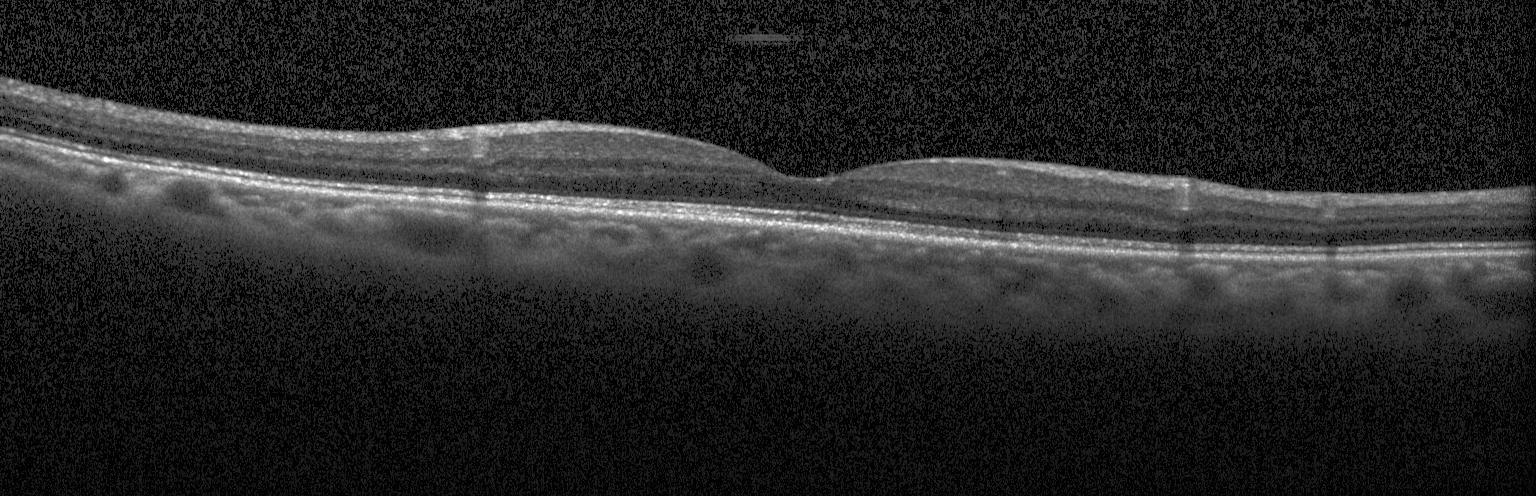 Spectral-domain OCT B-scan: no evidence of choroidal neovascularization, diabetic macular edema, or drusen.